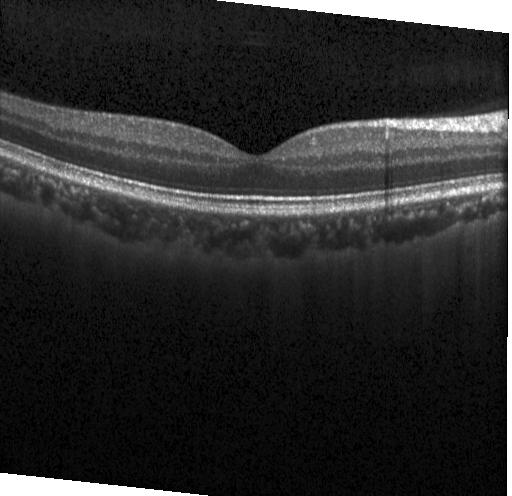

Impression: neither CNV, DME, nor drusen.